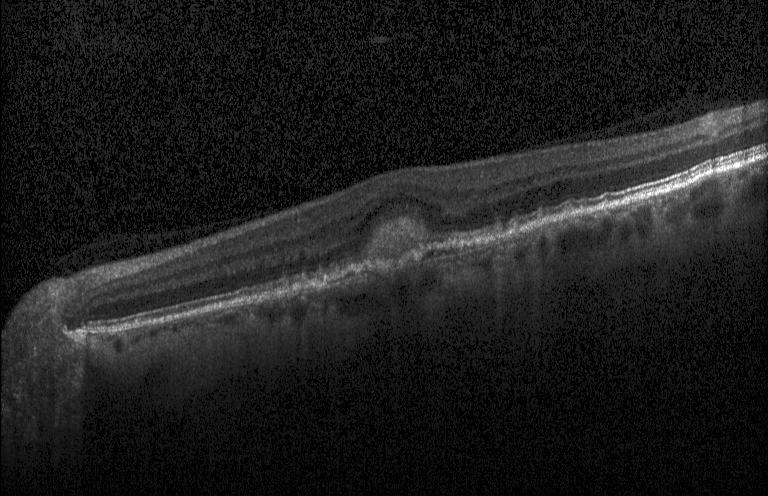 This B-scan demonstrates a choroidal neovascular membrane.